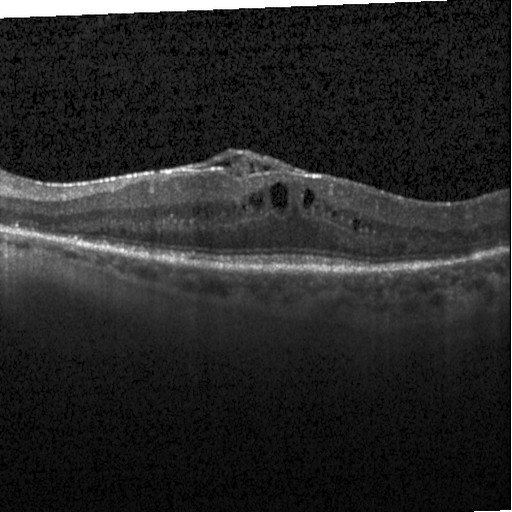
The scan shows diabetic macular edema.